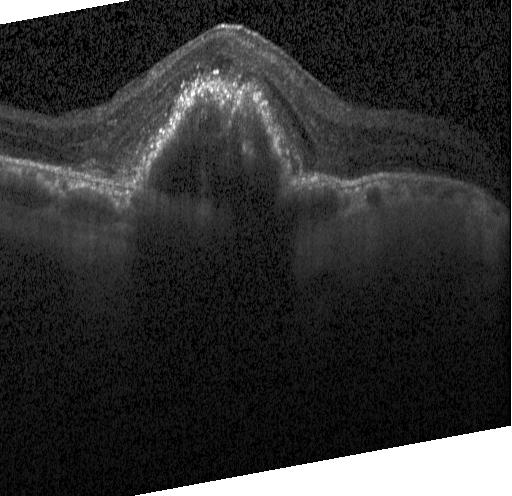

Macular scan, OCT line scan.
Finding: a choroidal neovascular membrane.